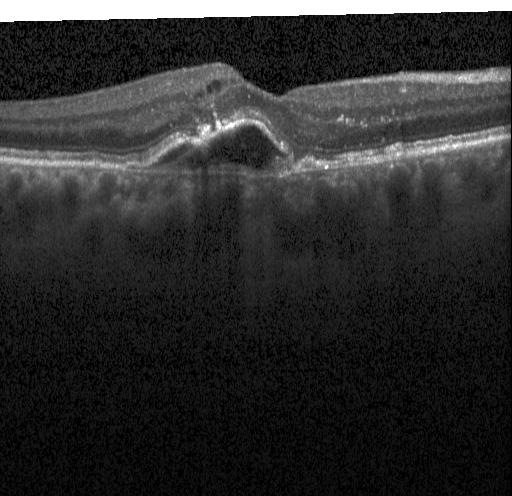
Heidelberg Spectralis OCT system · spectral-domain OCT · retinal OCT B-scan. Macular OCT: CNV.